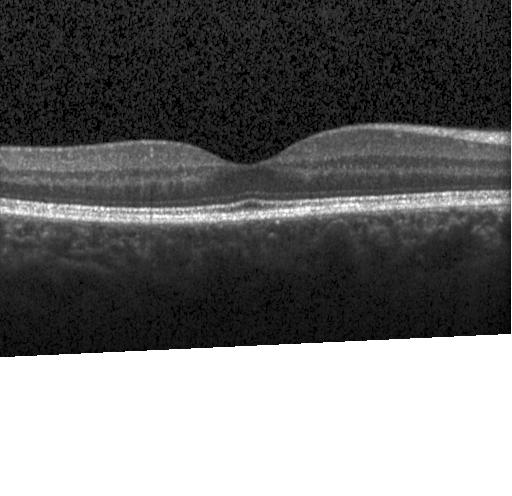 Acquired on a Heidelberg Spectralis, macular scan, OCT B-scan
Macular OCT: no choroidal neovascularization, diabetic macular edema, or drusen.